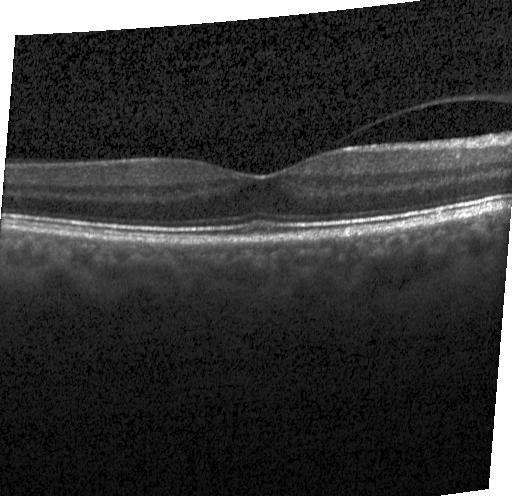

Spectral-domain optical coherence tomography. Retinal OCT B-scan. No CNV, DME, or drusen.